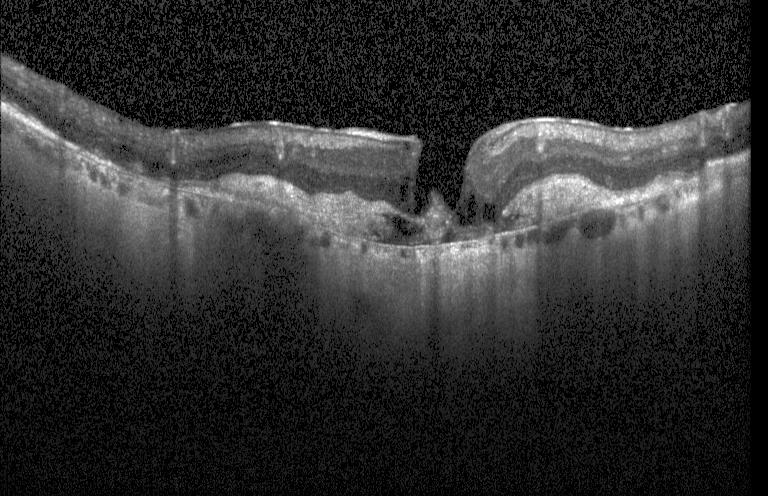
OCT B-scan showing CNV.